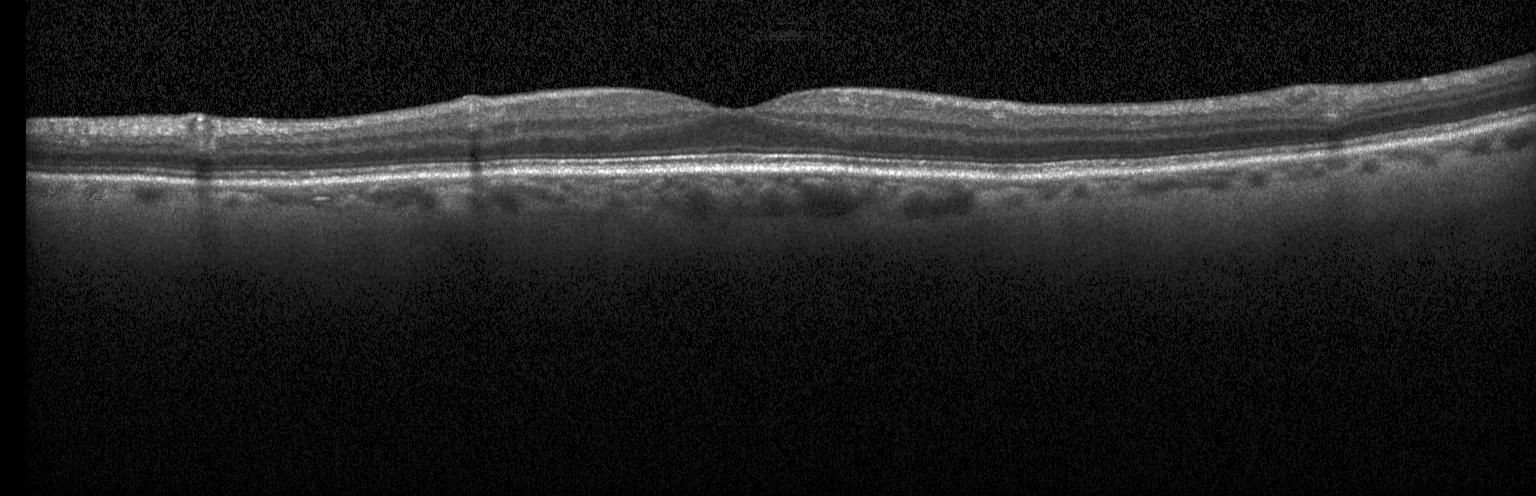

Impression: no CNV, no DME, and no drusen.